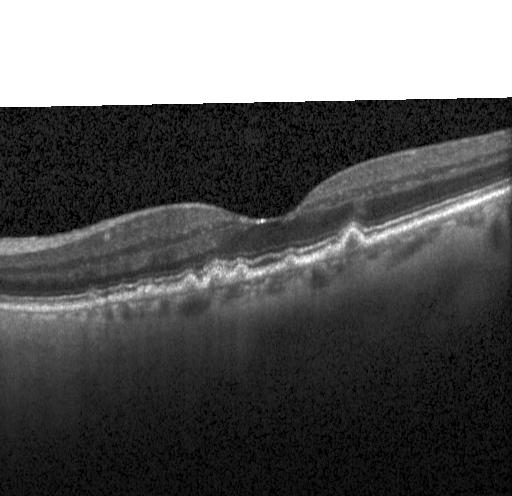
Centered on the fovea · retinal OCT B-scan — Finding: sub-RPE drusenoid deposits.